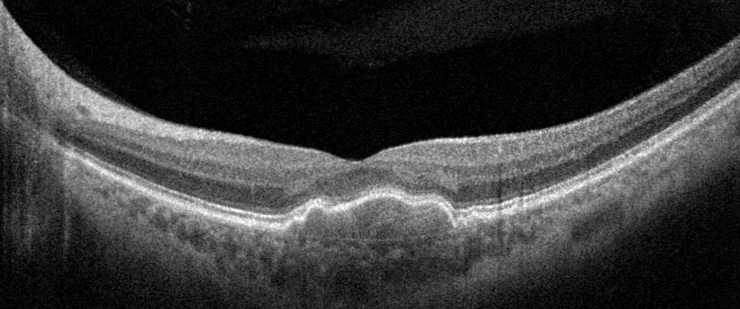

Through the macula, instrument: Optovue Avanti RTVue XR, retinal OCT cross-section. The scan shows AMD.